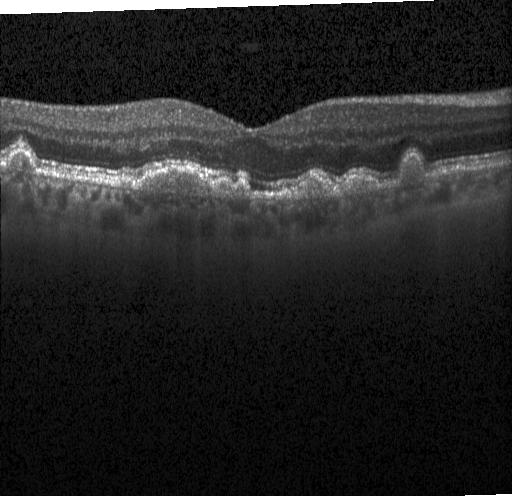 Optical coherence tomography B-scan · macular scan — Diagnosis: multiple drusen.